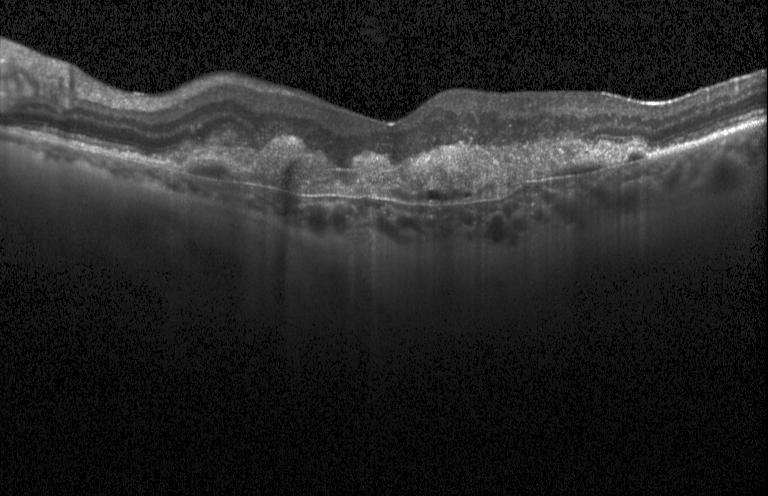
OCT B-scan, Heidelberg Spectralis, SD-OCT, centered on the fovea — CNV.